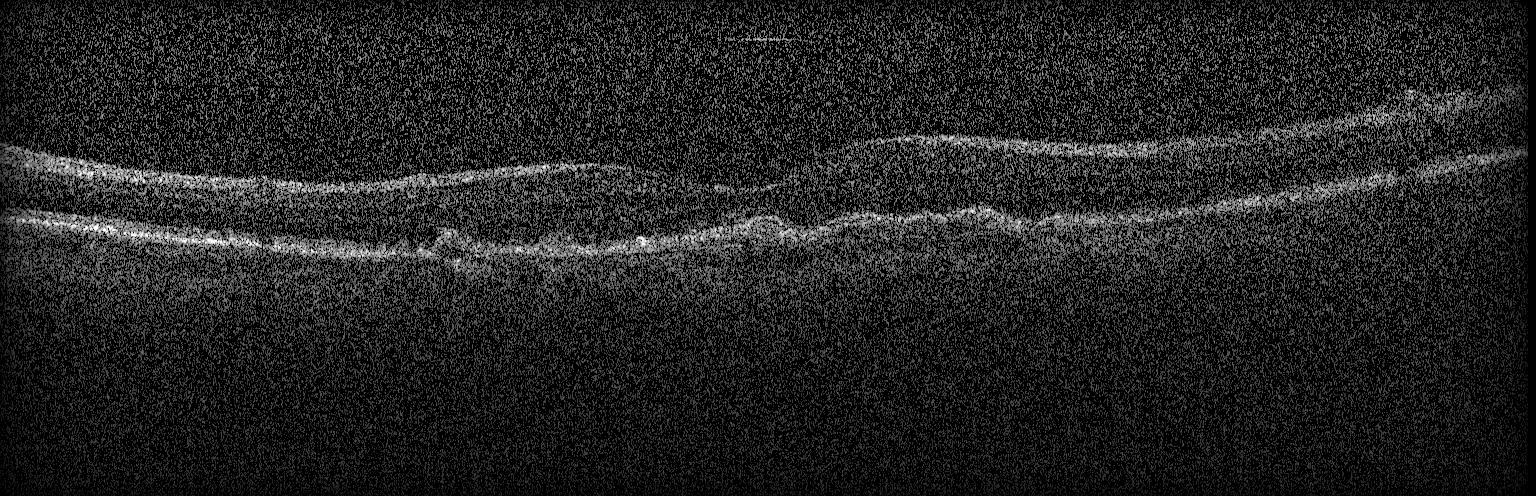 Impression: choroidal neovascularization (CNV).